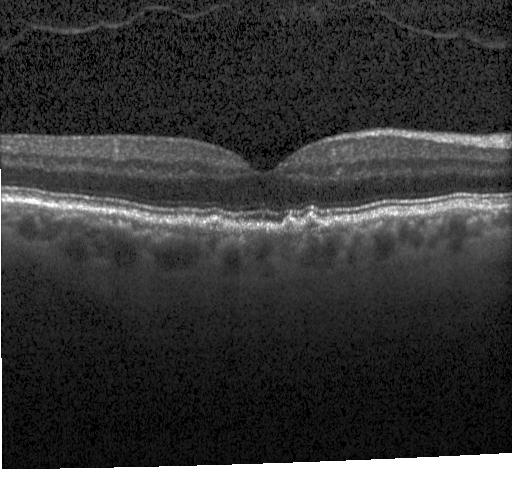 Retinal OCT cross-section, SD-OCT, Heidelberg Spectralis. Diagnosis: drusen.